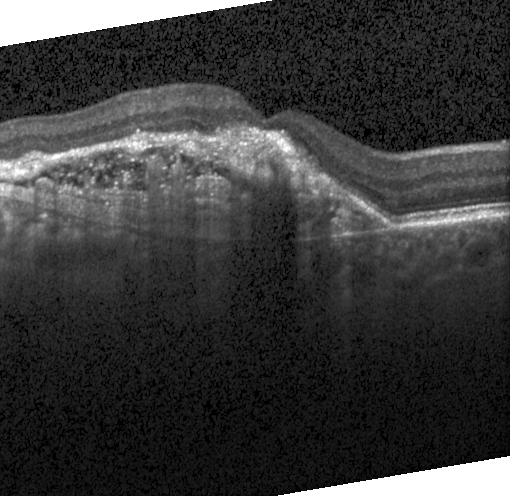 Retinal OCT cross-section · centered on the fovea.
Macular OCT: choroidal neovascularization (CNV).